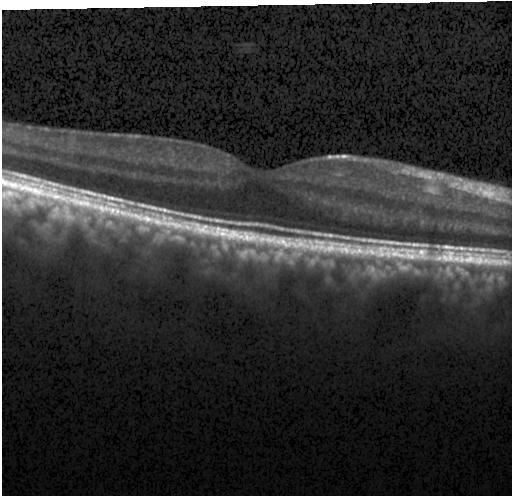

Macular scan. Retinal OCT cross-section. Finding: no choroidal neovascularization, diabetic macular edema, or drusen.